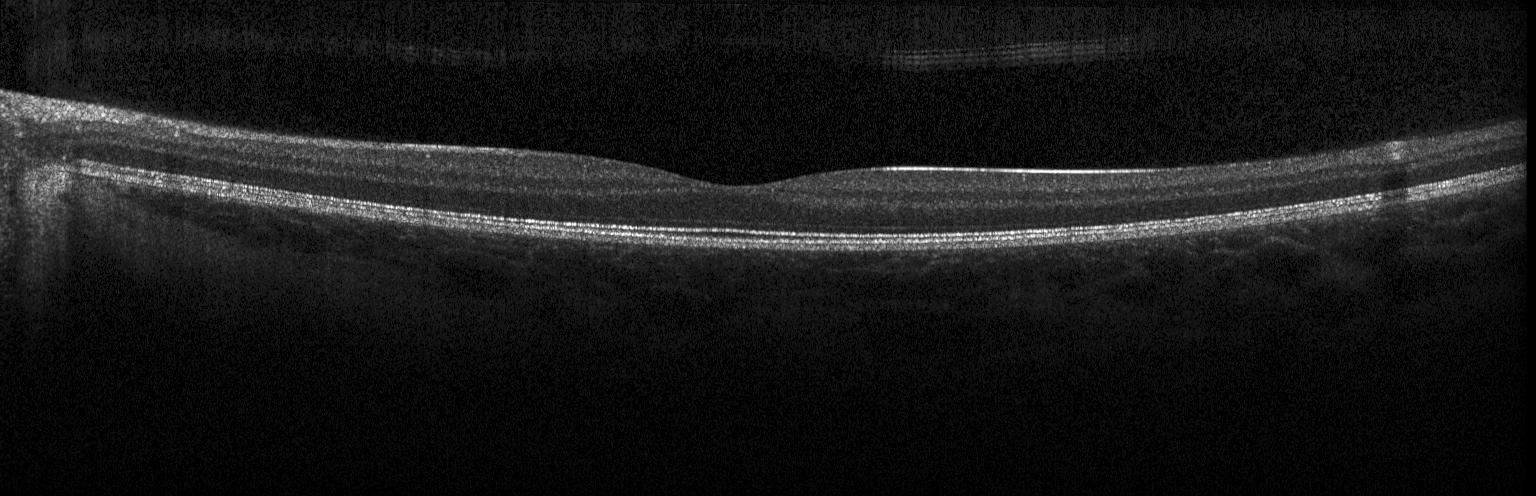
Finding: neither choroidal neovascularization, diabetic macular edema, nor drusen.